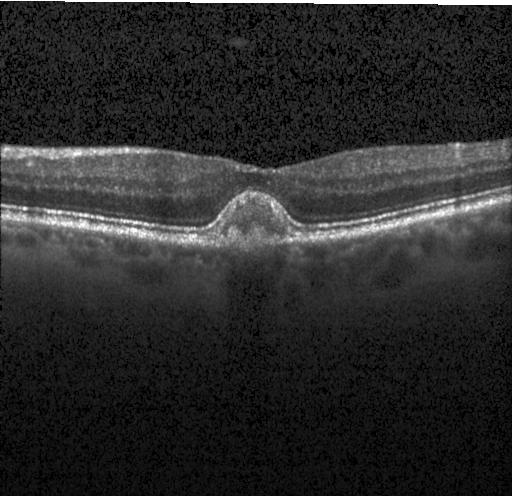

Retinal OCT cross-section showing CNV.